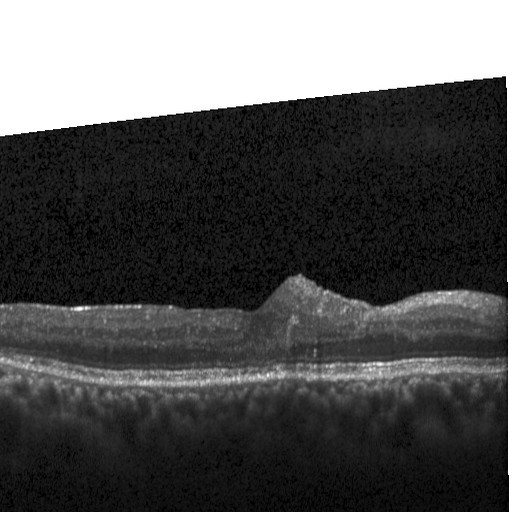
This B-scan demonstrates diabetic macular edema (DME).